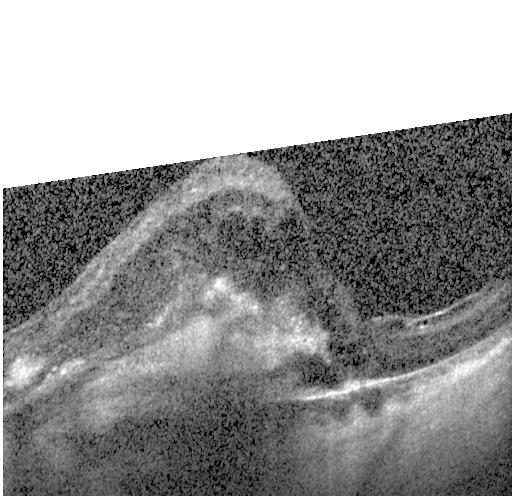
Diagnosis: CNV.